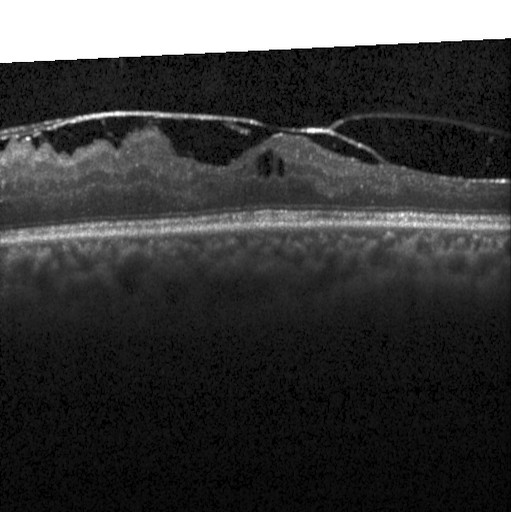 Impression: diabetic macular edema.